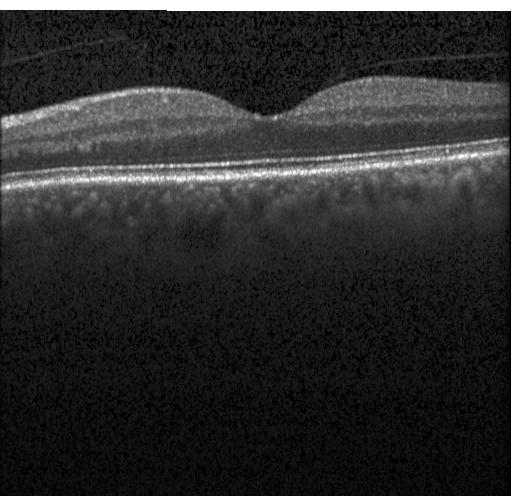
Spectral-domain optical coherence tomography · optical coherence tomography scan — OCT finding: no choroidal neovascularization, no diabetic macular edema, and no drusen.